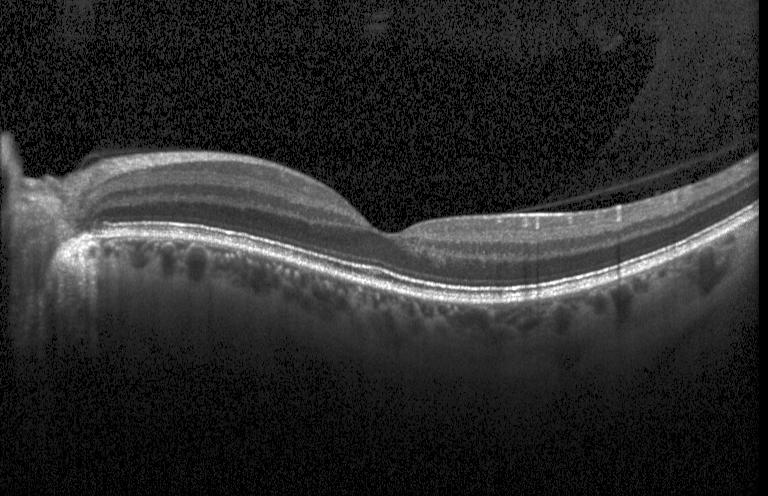
OCT finding: no evidence of choroidal neovascularization, diabetic macular edema, or drusen.